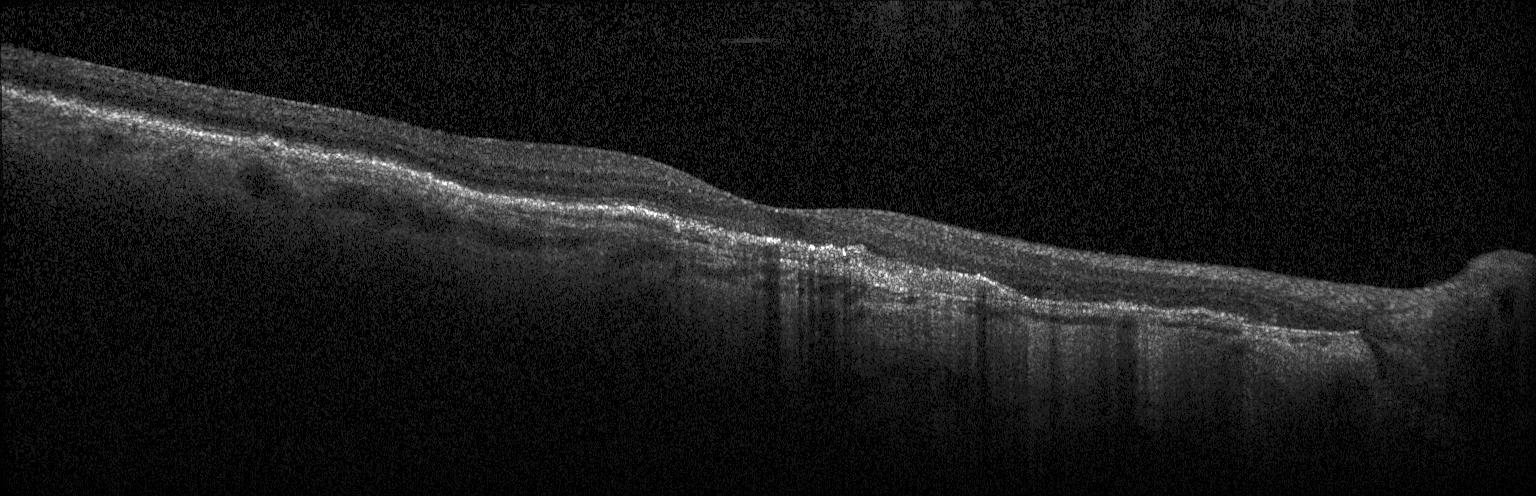
Assessment: choroidal neovascularization.